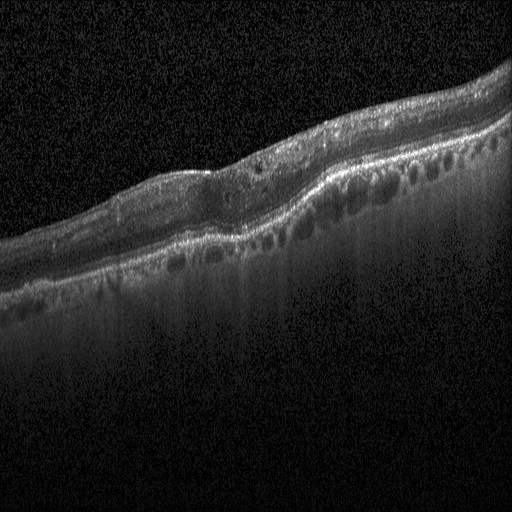

Finding: DME.